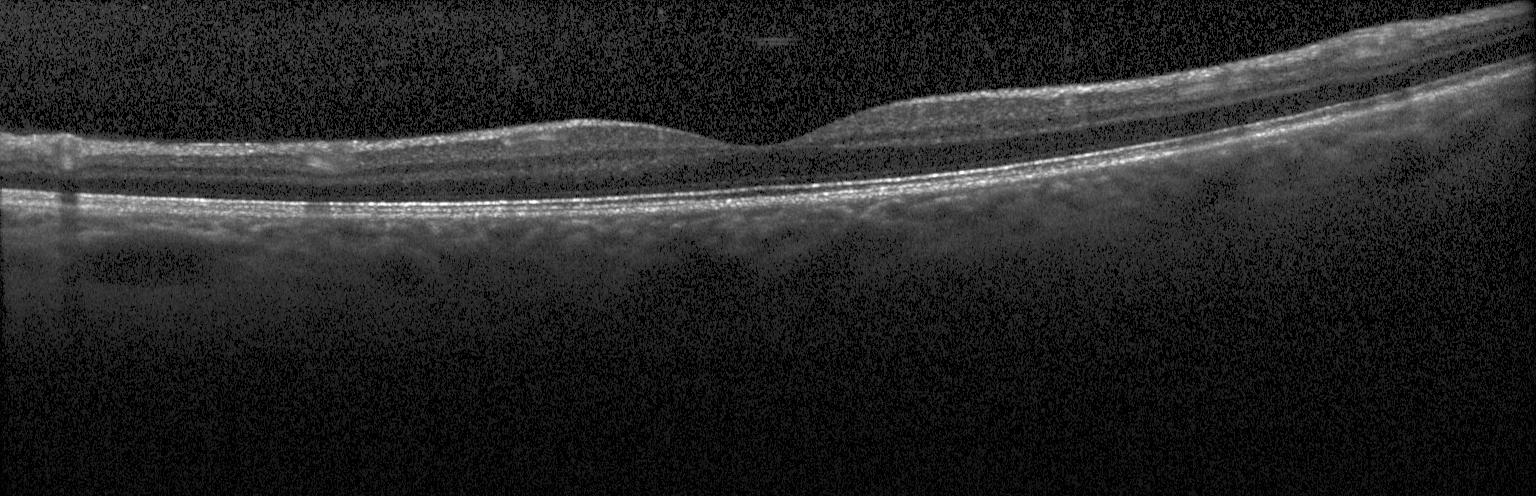

No choroidal neovascularization, no diabetic macular edema, and no drusen.